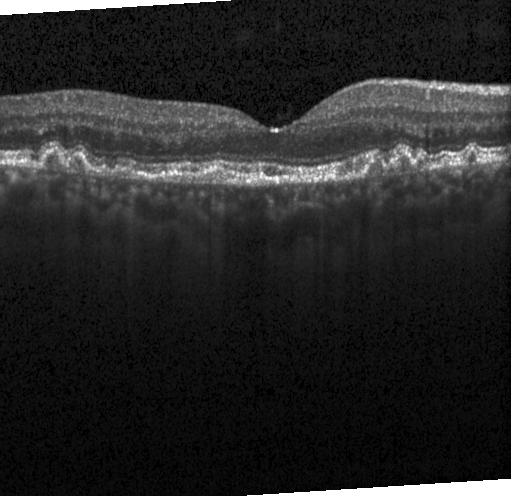 Through the macula; OCT B-scan; spectral-domain optical coherence tomography — Diagnosis: sub-RPE drusenoid deposits.